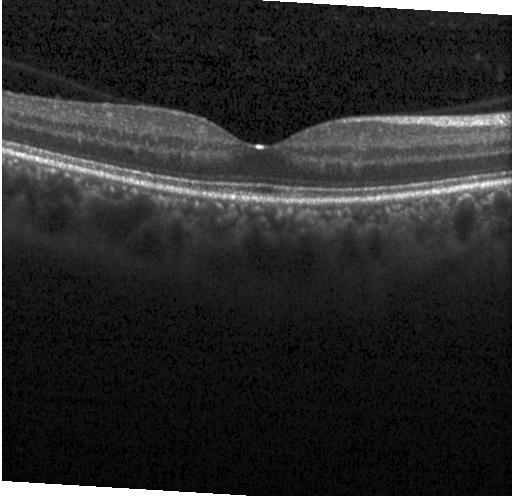

Horizontal scan through the fovea, SD-OCT, retinal OCT cross-section — No choroidal neovascularization, diabetic macular edema, or drusen.